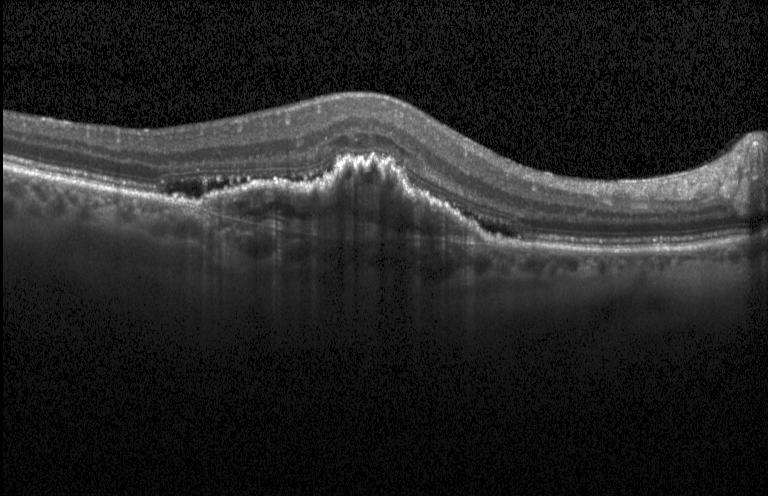 Macular OCT: a choroidal neovascular membrane.